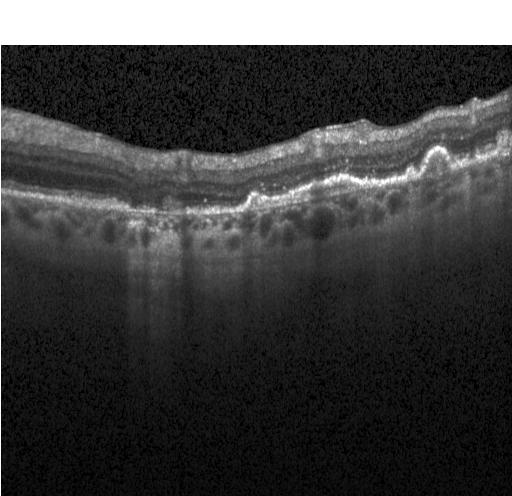
Heidelberg Spectralis, retinal OCT cross-section
Impression: choroidal neovascularization (CNV).